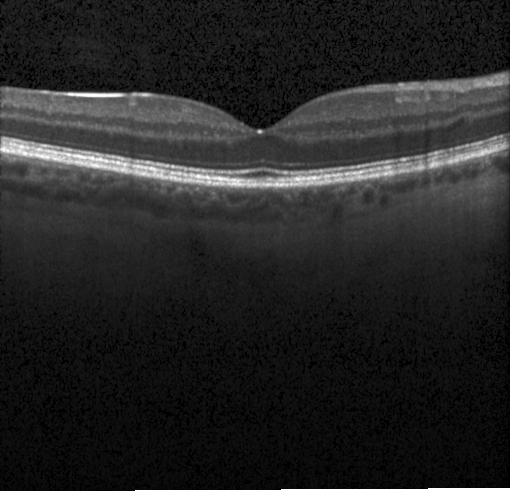 Impression: no evidence of CNV, DME, or drusen.